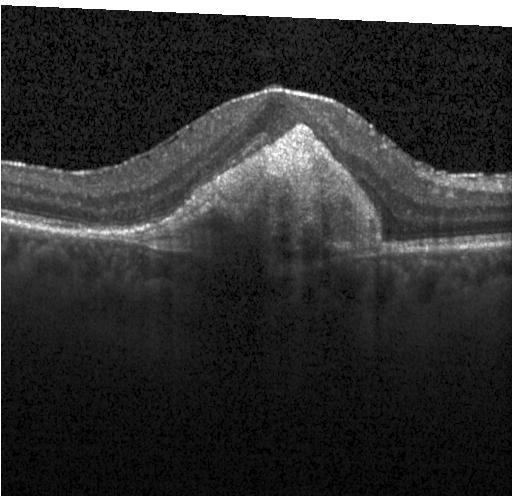 Spectral-domain optical coherence tomography. Horizontal scan through the fovea. Heidelberg Spectralis. Optical coherence tomography scan — The scan shows choroidal neovascularization.